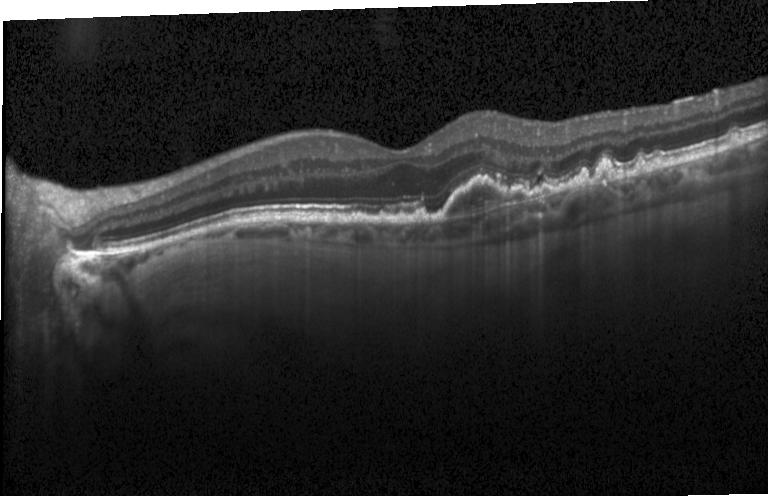

Optical coherence tomography B-scan. Macular scan. This B-scan demonstrates a choroidal neovascular membrane.